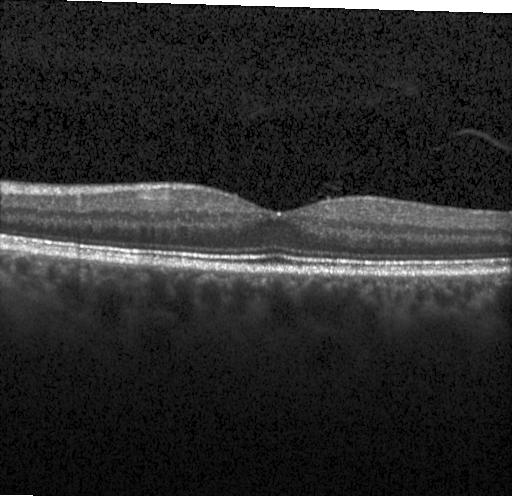

This B-scan demonstrates no choroidal neovascularization, diabetic macular edema, or drusen.